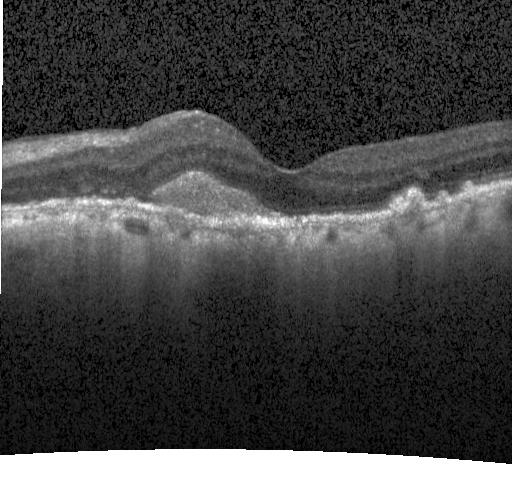
Spectral-domain OCT; acquired on a Heidelberg Spectralis; centered on the fovea; optical coherence tomography scan. Dx: CNV.